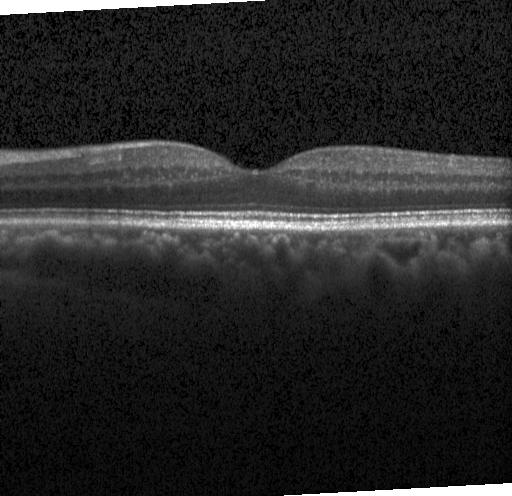
OCT B-scan. Macular scan. Acquired on a Heidelberg Spectralis. Spectral-domain OCT.
Macular OCT: no evidence of CNV, DME, or drusen.